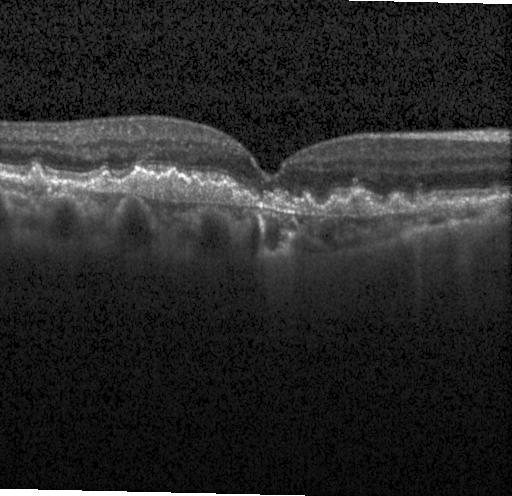 Spectral-domain OCT. Optical coherence tomography B-scan. Acquired on a Heidelberg Spectralis.
Choroidal neovascularization.